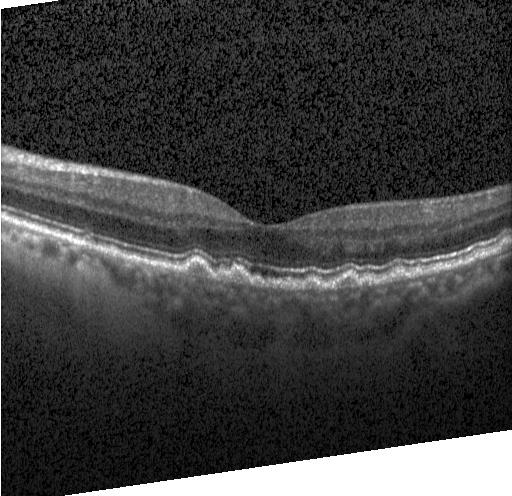
Centered on the fovea · acquired on a Heidelberg Spectralis · retinal OCT cross-section · spectral-domain OCT. Diagnosis: multiple drusen.